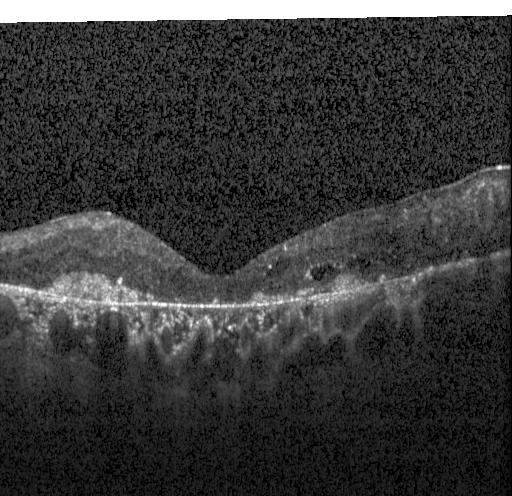
Impression: a choroidal neovascular membrane.